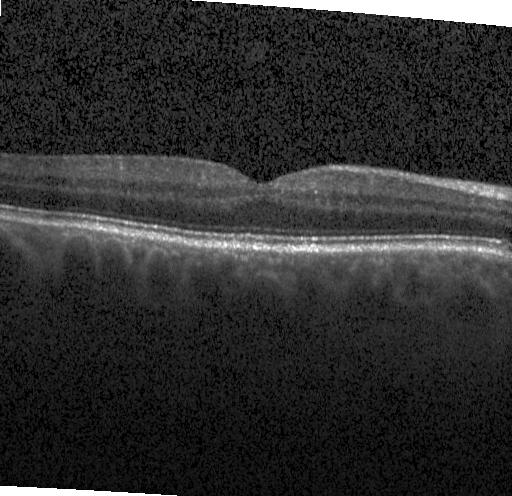
OCT B-scan showing no choroidal neovascularization, no diabetic macular edema, and no drusen.